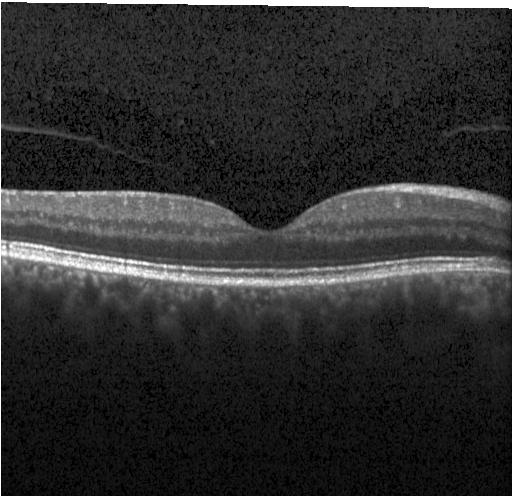 Optical coherence tomography scan. Acquired on a Heidelberg Spectralis. Macular scan
Diagnosis: no CNV, no DME, and no drusen.